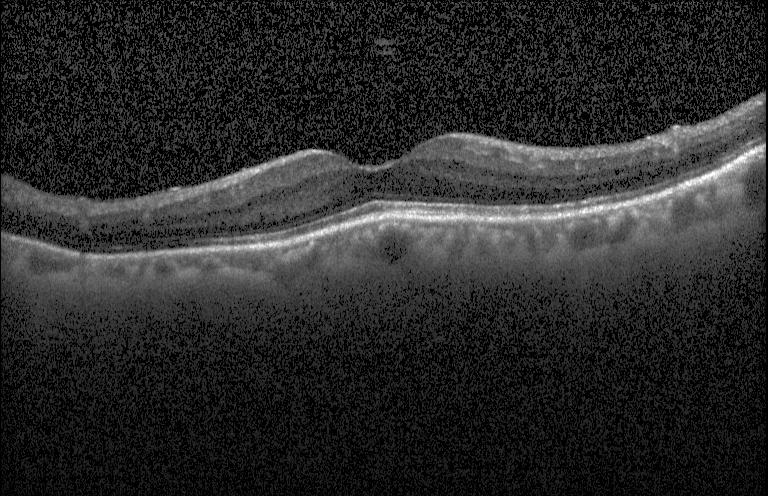
Spectral-domain OCT B-scan: neither choroidal neovascularization, diabetic macular edema, nor drusen.